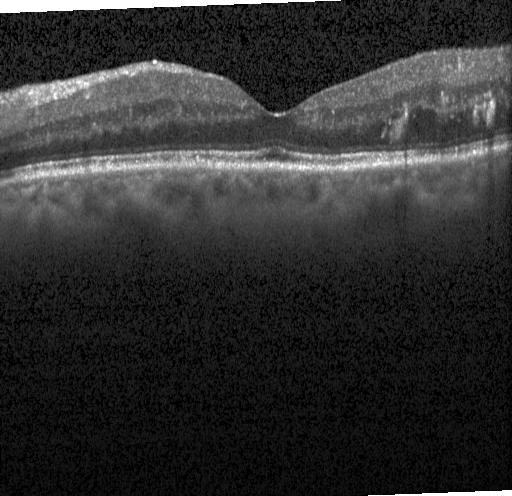 Macular OCT: DME.